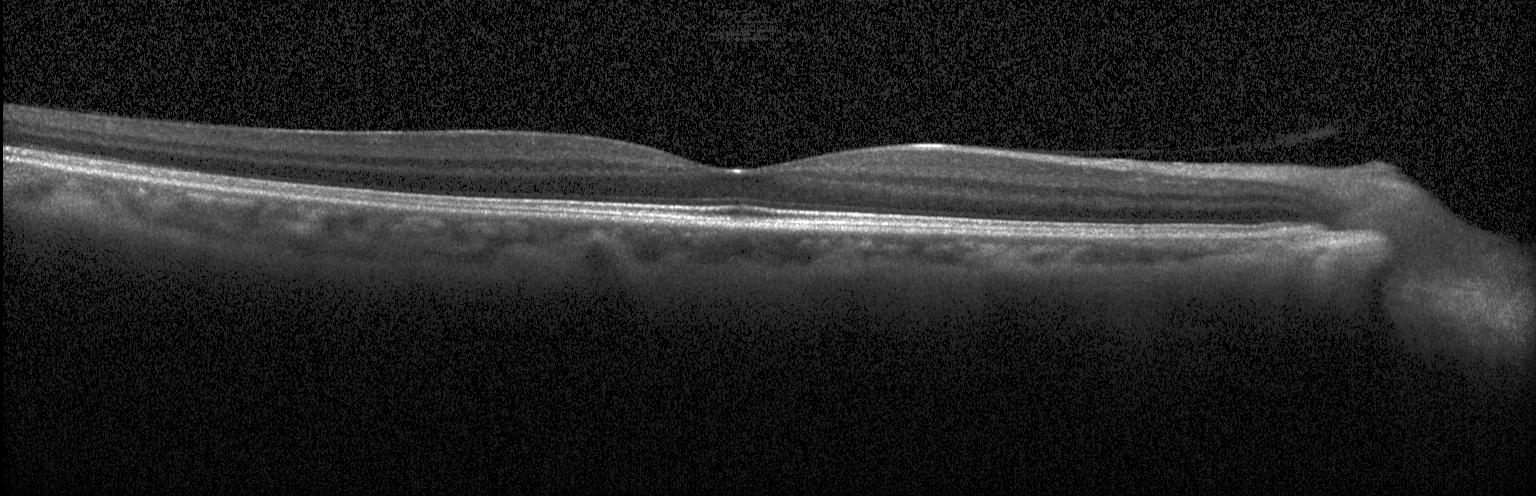
The scan shows neither choroidal neovascularization, diabetic macular edema, nor drusen.